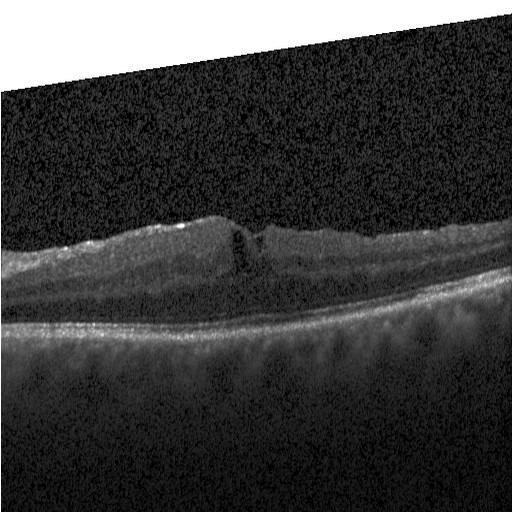 Spectral-domain optical coherence tomography. Fovea-centered. Acquired on a Heidelberg Spectralis. Retinal OCT B-scan. Impression: DME.